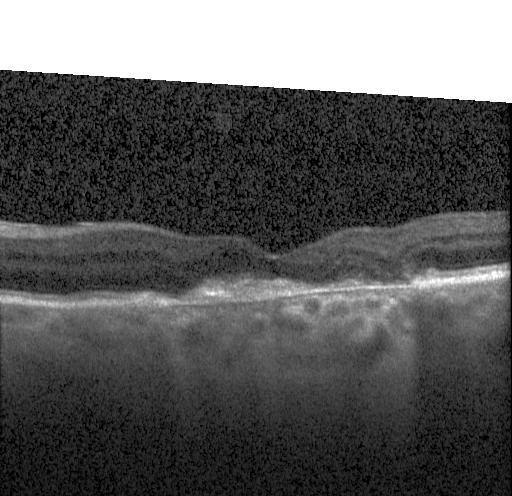 Spectral-domain optical coherence tomography; acquired on a Heidelberg Spectralis; OCT line scan — Dx: choroidal neovascularization (CNV).